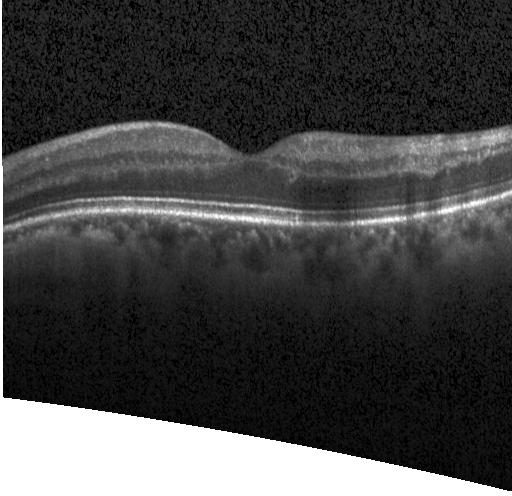
OCT scan showing no evidence of choroidal neovascularization, diabetic macular edema, or drusen.